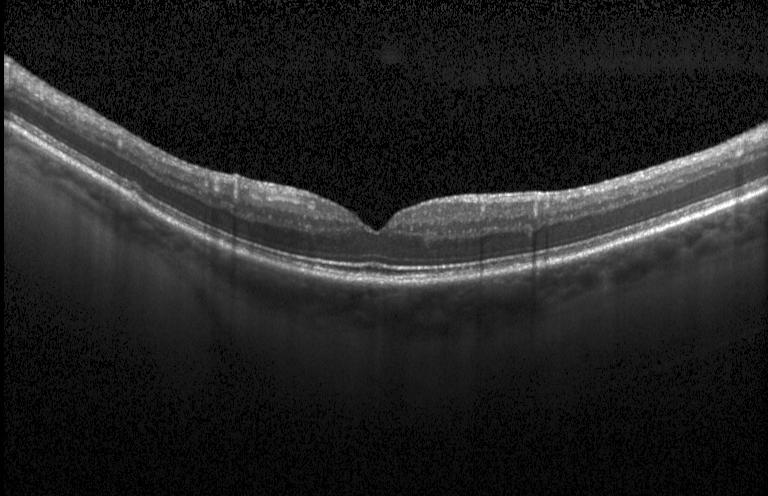
This B-scan demonstrates neither choroidal neovascularization, diabetic macular edema, nor drusen.